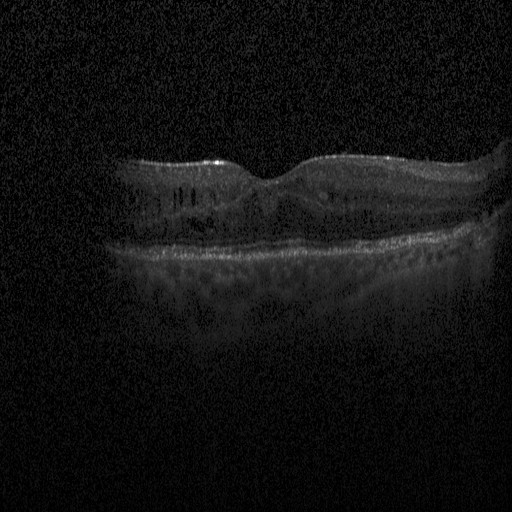
Spectral-domain optical coherence tomography, optical coherence tomography B-scan
This B-scan demonstrates diabetic macular edema.